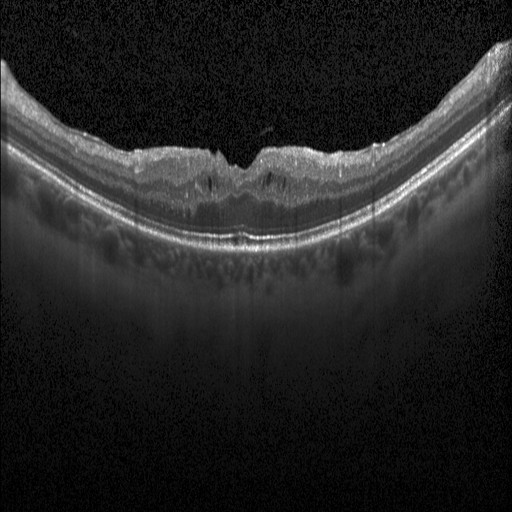

OCT line scan.
Assessment: diabetic macular edema.